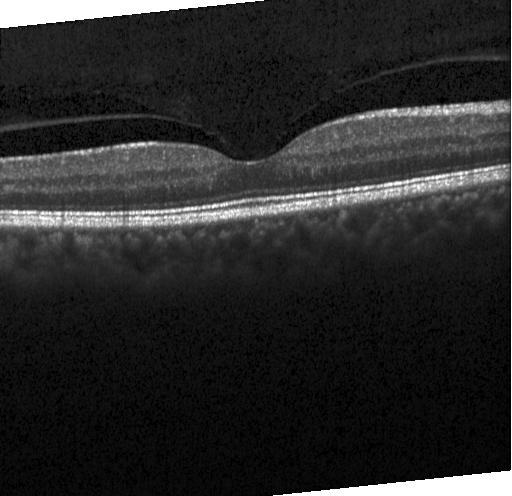 Macular OCT: no evidence of choroidal neovascularization, diabetic macular edema, or drusen.